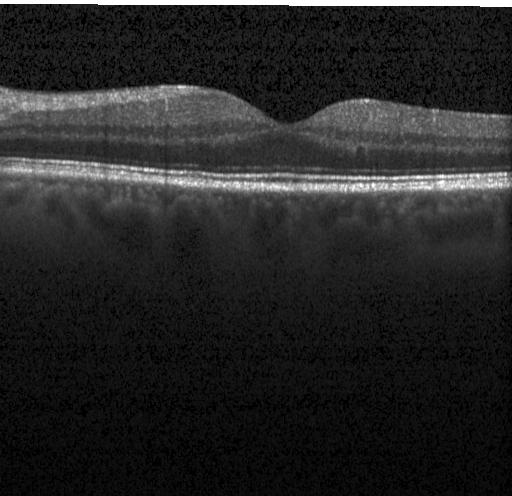

Diagnosis: no evidence of CNV, DME, or drusen.